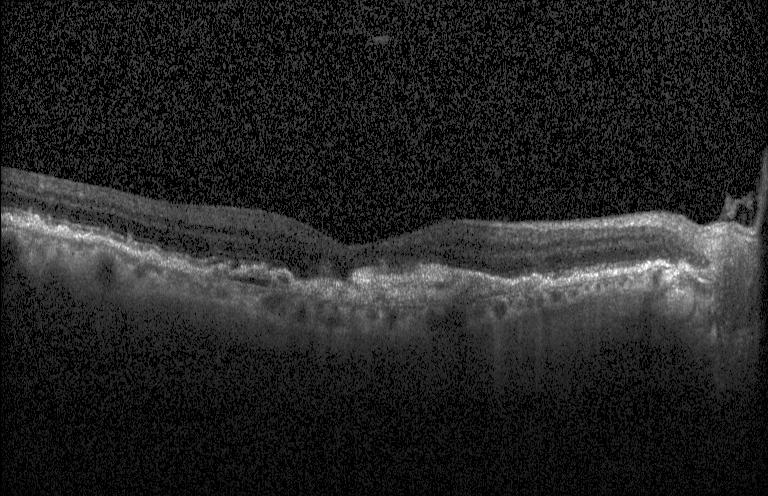

Diagnosis: a choroidal neovascular membrane.